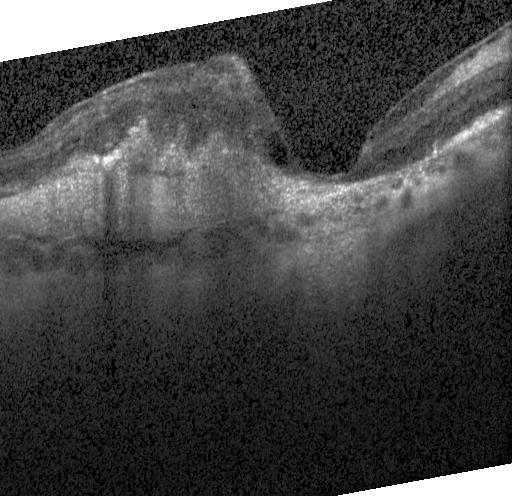 OCT line scan — Dx: choroidal neovascularization.